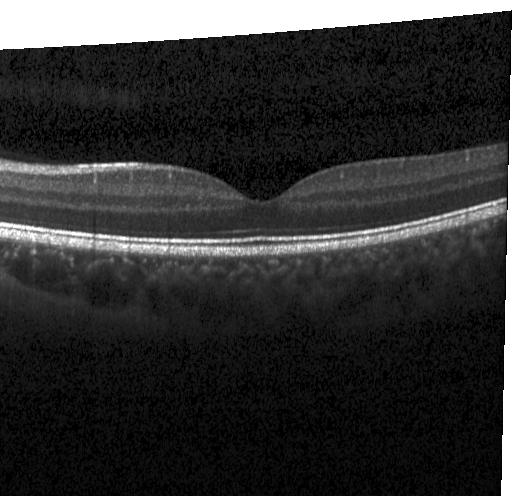 Fovea-centered · optical coherence tomography scan.
No evidence of choroidal neovascularization, diabetic macular edema, or drusen.